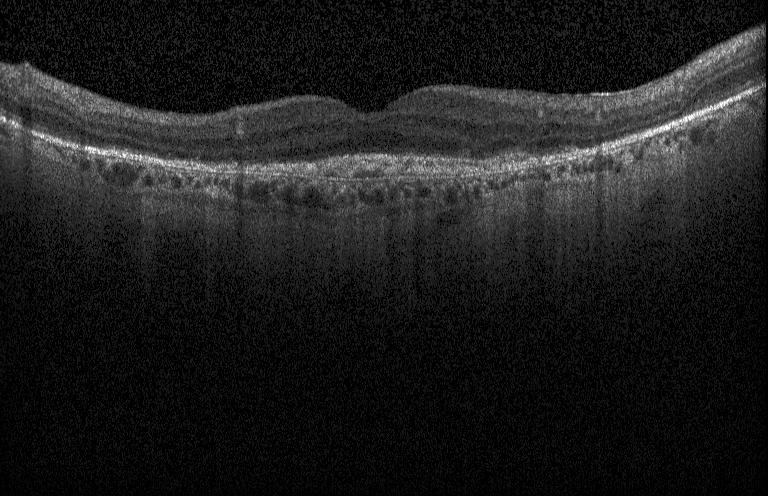

Retinal OCT cross-section, through the macula, Heidelberg Spectralis. Diagnosis: a choroidal neovascular membrane.